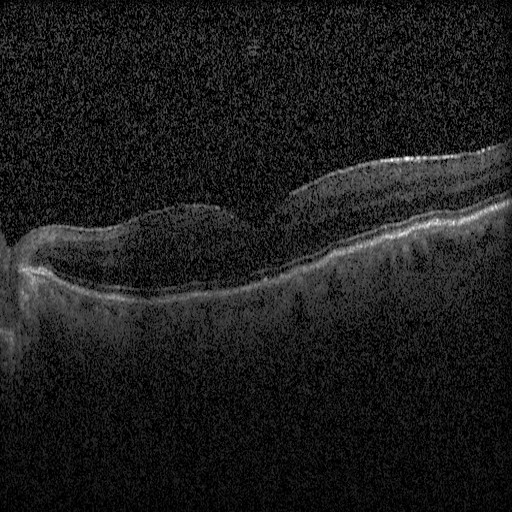 Horizontal scan through the fovea · retinal OCT B-scan · spectral-domain OCT.
Finding: DME.